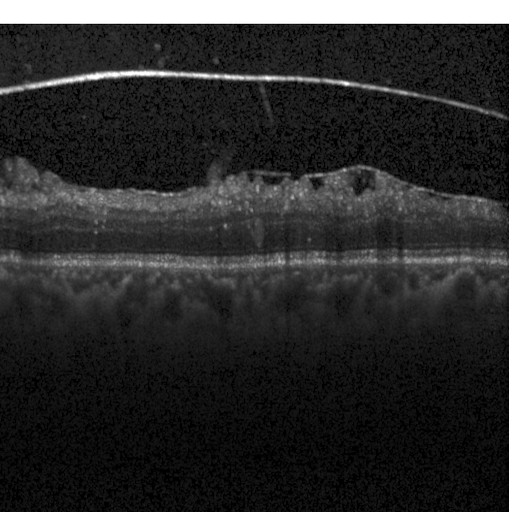

SD-OCT; OCT B-scan; acquired on a Heidelberg Spectralis. Finding: DME.